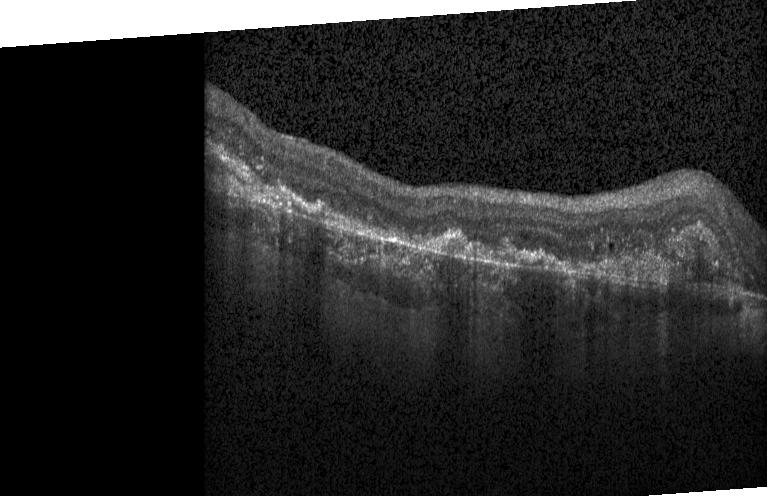
OCT B-scan showing a choroidal neovascular membrane.